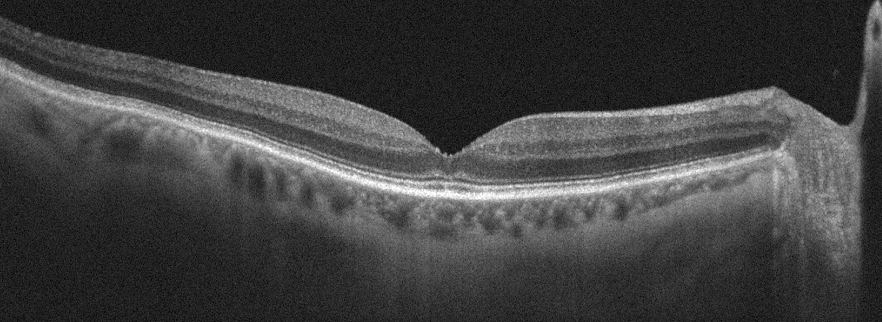
OD; optical coherence tomography scan; fovea-centered — Absence of AMD, DME, ERM, RAO, RVO, and vitreomacular interface disease.